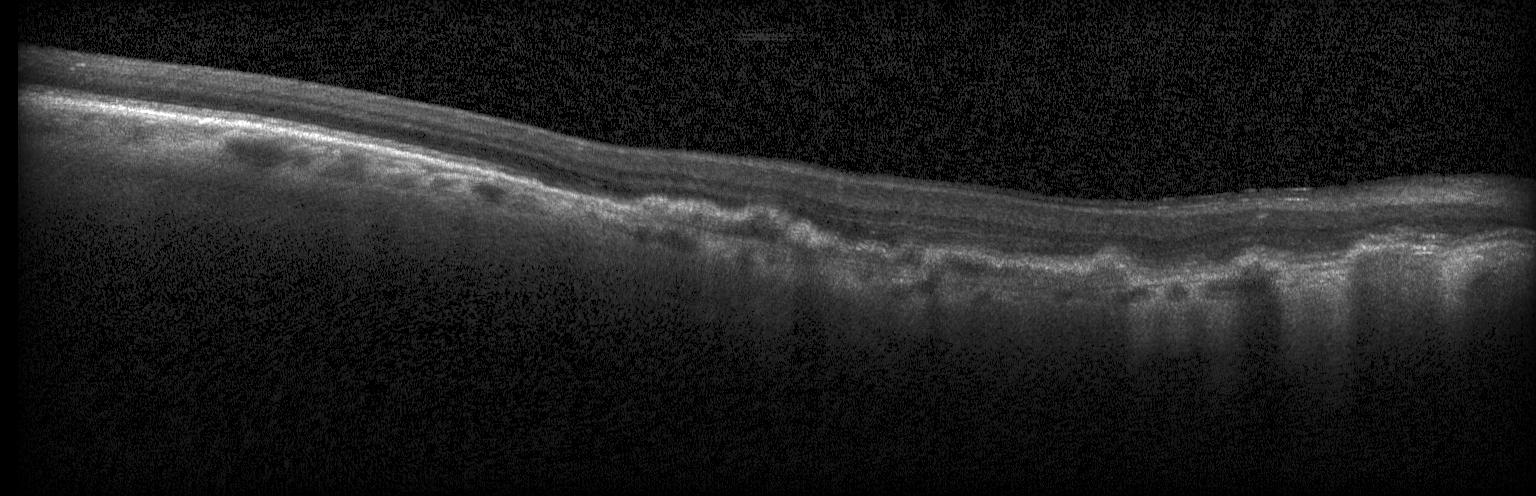
SD-OCT. OCT B-scan
OCT finding: a choroidal neovascular membrane.